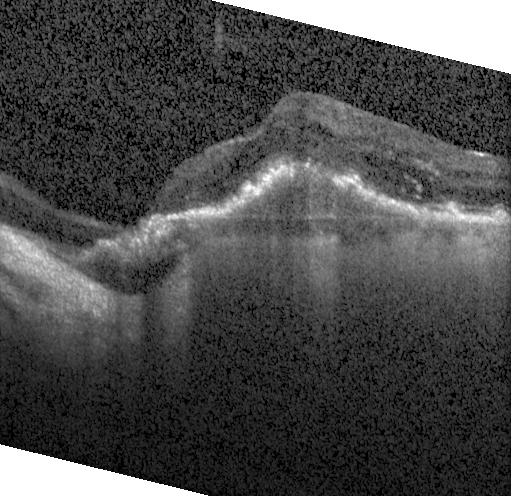 Assessment: choroidal neovascularization (CNV).